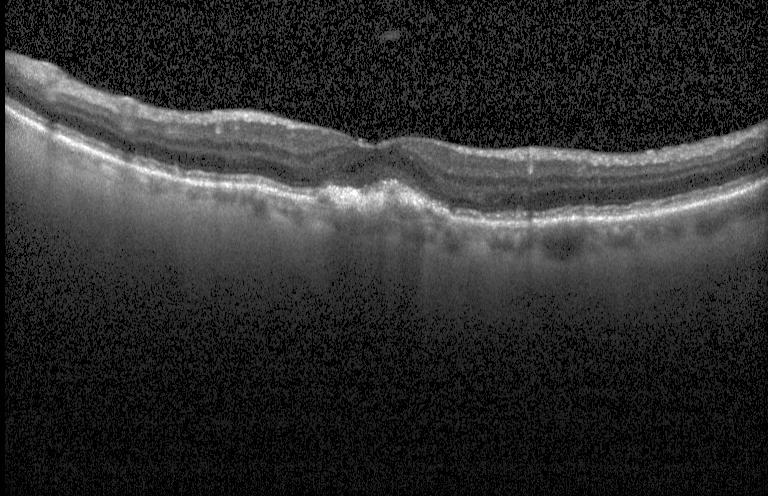 OCT B-scan — Finding: choroidal neovascularization (CNV).